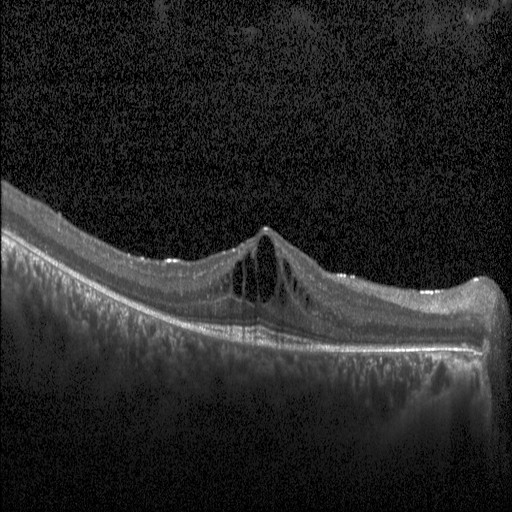 Optical coherence tomography scan
Dx: DME.